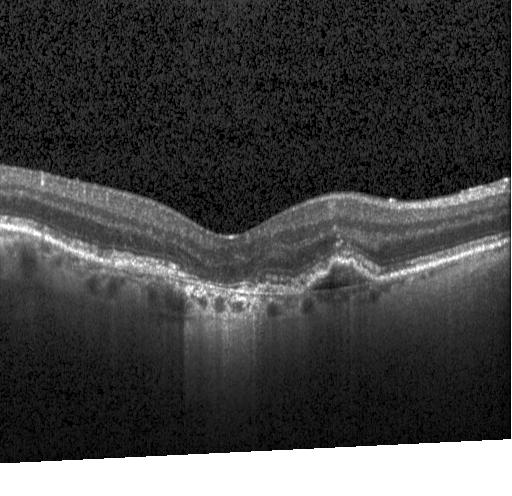

Heidelberg Spectralis · OCT line scan · SD-OCT. Dx: choroidal neovascularization (CNV).